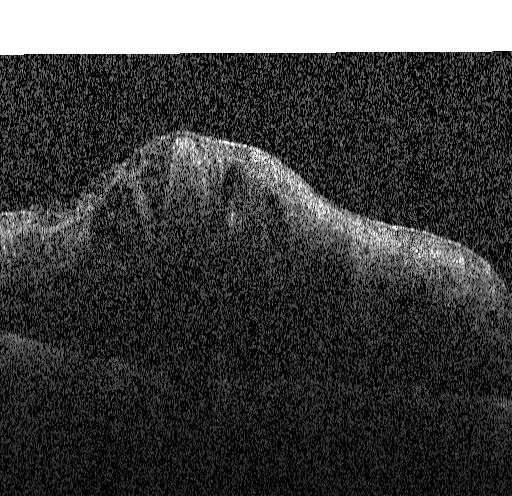 Retinal OCT B-scan · instrument: Heidelberg Spectralis — Finding: DME.